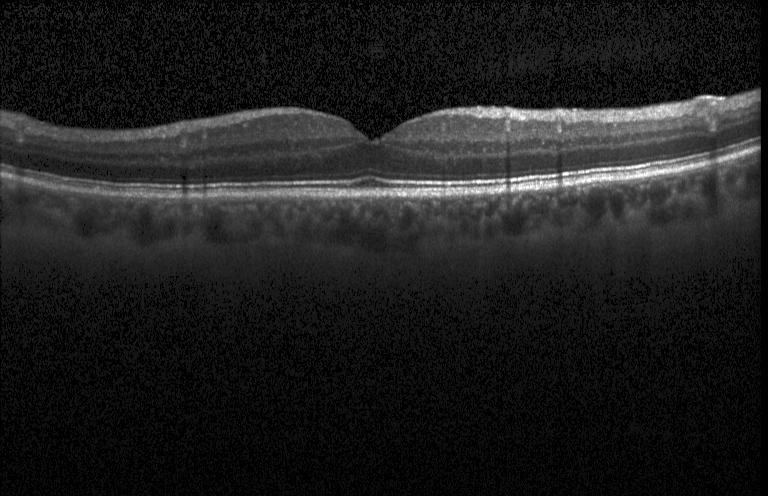 Finding: no choroidal neovascularization, diabetic macular edema, or drusen.